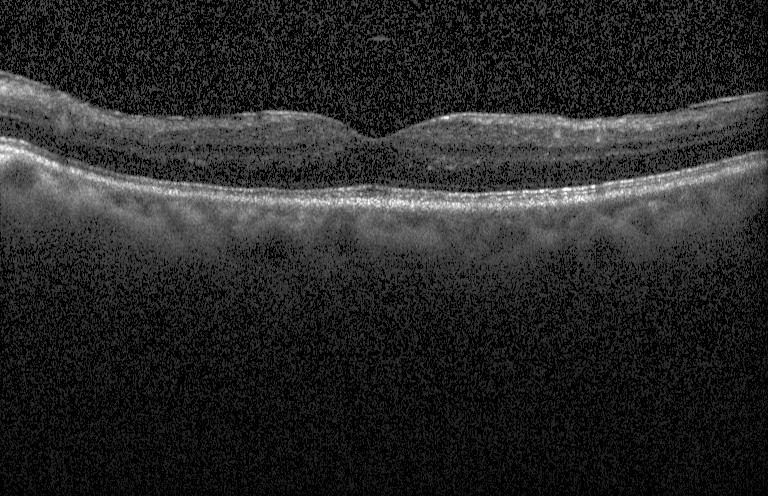 Diagnosis: no choroidal neovascularization, diabetic macular edema, or drusen.